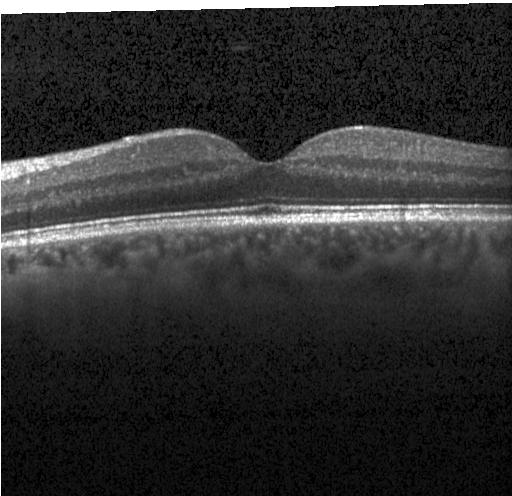

Retinal OCT cross-section showing no choroidal neovascularization, diabetic macular edema, or drusen.